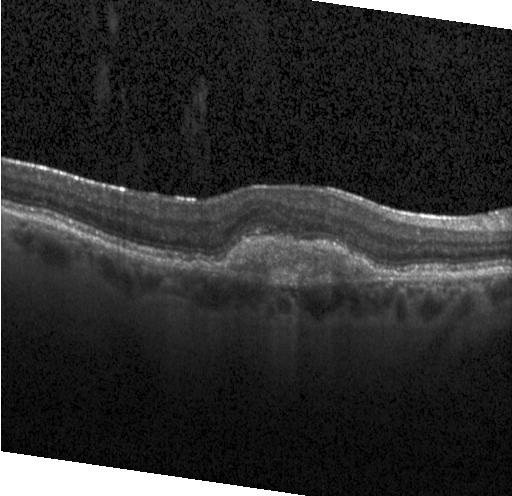 Instrument: Heidelberg Spectralis; fovea-centered; SD-OCT; optical coherence tomography scan.
Choroidal neovascularization.